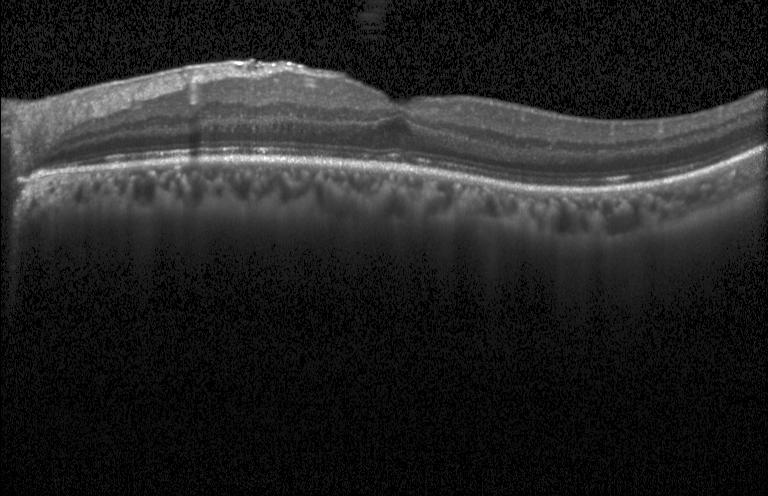 Optical coherence tomography scan. Macular OCT: no choroidal neovascularization, diabetic macular edema, or drusen.